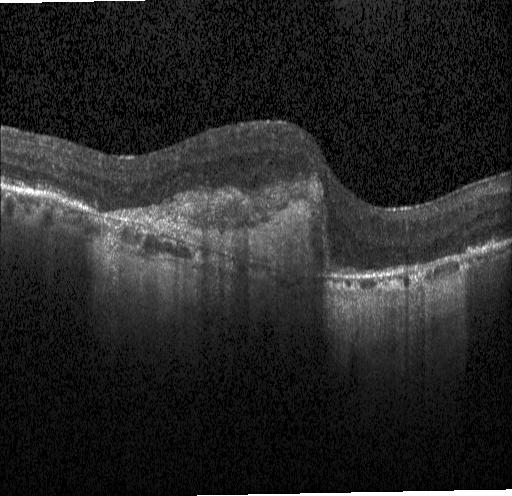 OCT line scan · Heidelberg Spectralis OCT system · macular scan · SD-OCT
Finding: a choroidal neovascular membrane.